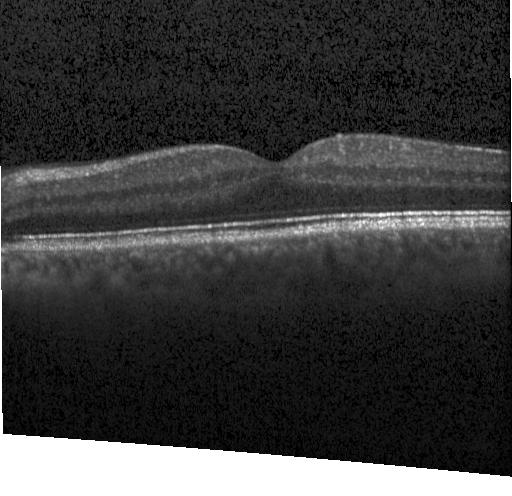

SD-OCT; OCT line scan. This B-scan demonstrates no choroidal neovascularization, diabetic macular edema, or drusen.